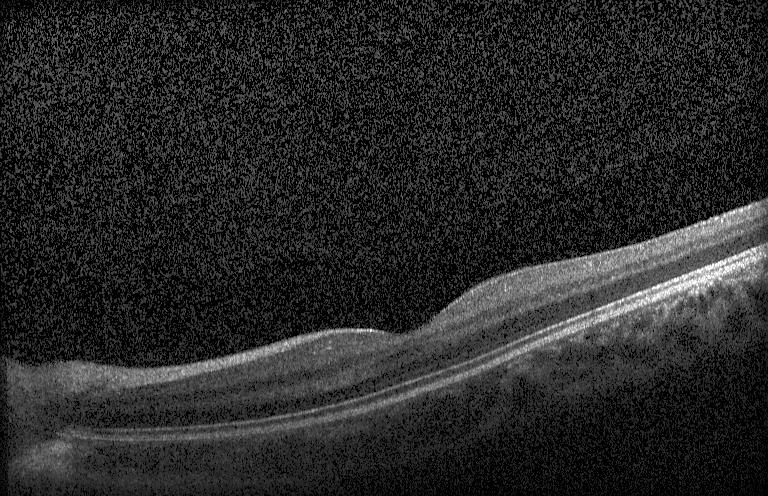 Finding: no CNV, DME, or drusen.